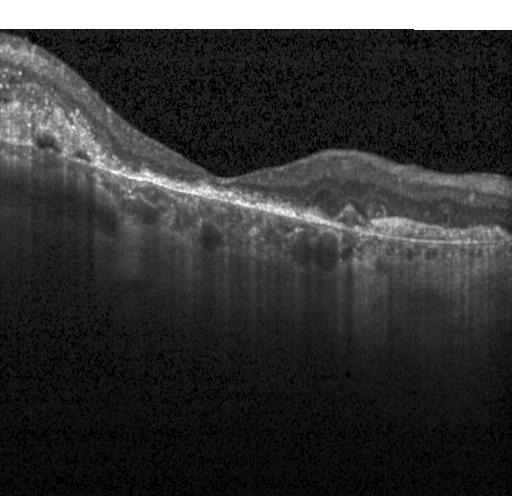
Instrument: Heidelberg Spectralis. OCT line scan. OCT finding: a choroidal neovascular membrane.